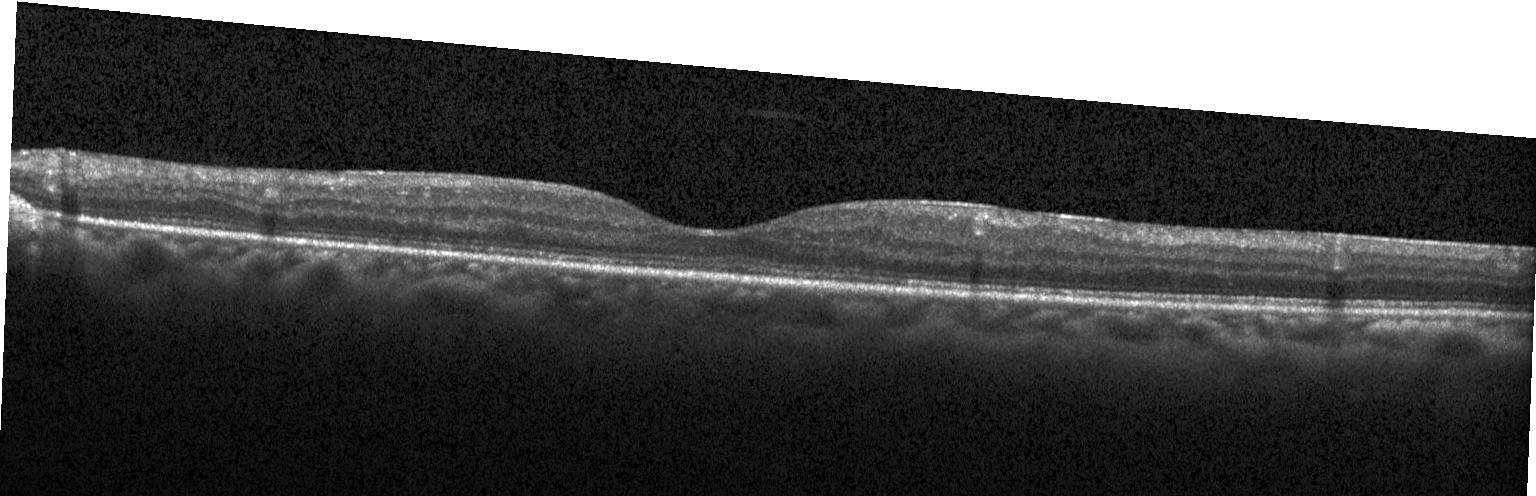 Through the macula; optical coherence tomography scan; SD-OCT.
Finding: neither choroidal neovascularization, diabetic macular edema, nor drusen.